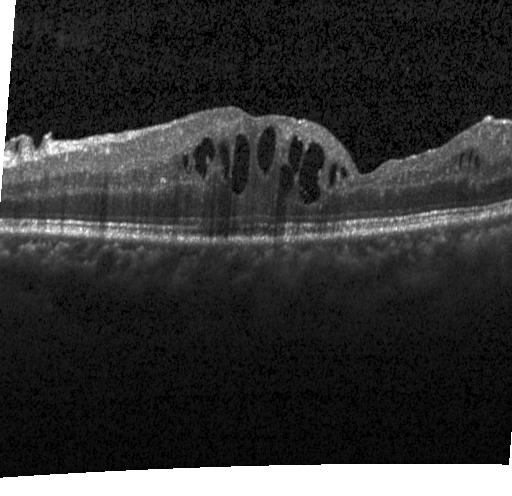 Horizontal scan through the fovea, optical coherence tomography scan. Dx: diabetic macular edema.